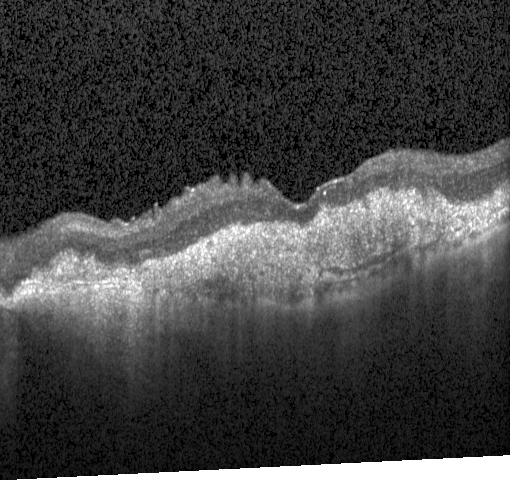
Optical coherence tomography scan.
Assessment: choroidal neovascularization (CNV).